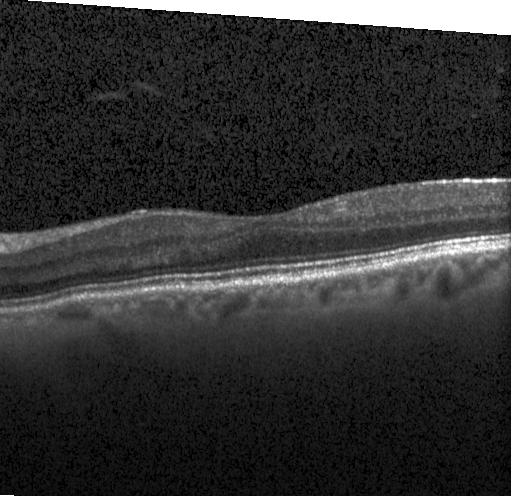
Optical coherence tomography B-scan · SD-OCT — Finding: no evidence of choroidal neovascularization, diabetic macular edema, or drusen.